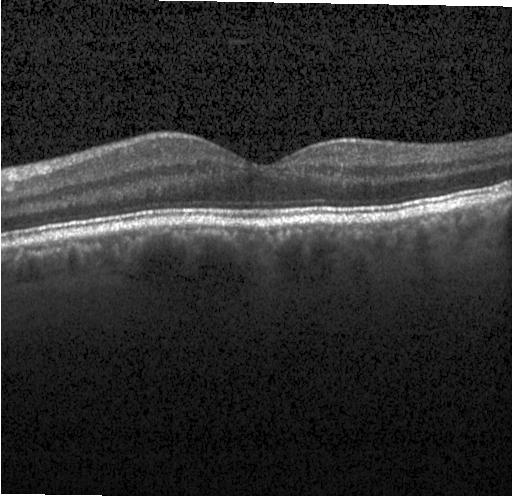
OCT scan showing no evidence of CNV, DME, or drusen.